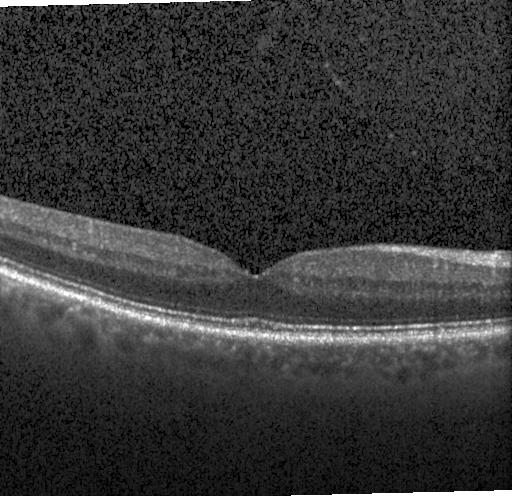

Through the macula · retinal OCT B-scan.
No CNV, DME, or drusen.